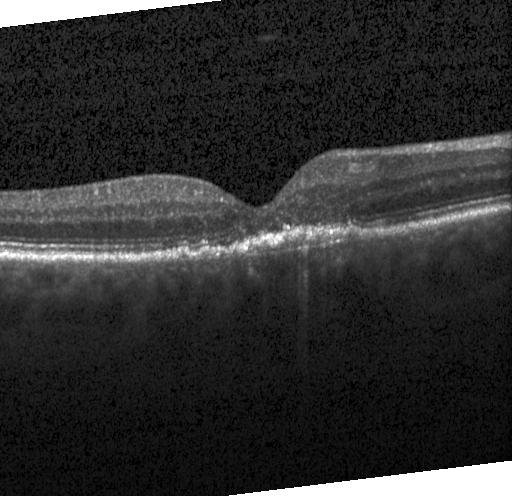 Assessment: a choroidal neovascular membrane.